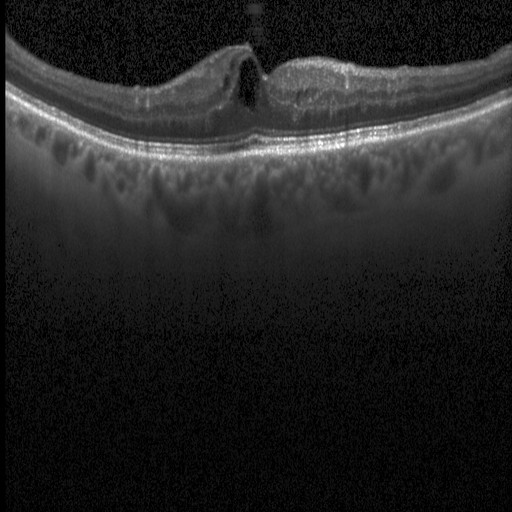 Optical coherence tomography B-scan.
OCT finding: diabetic macular edema.